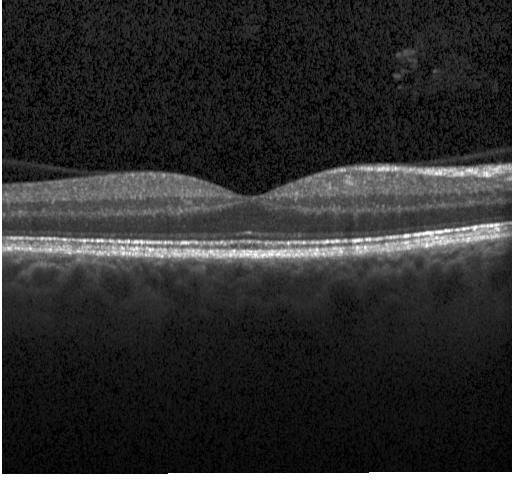 Instrument: Heidelberg Spectralis. Spectral-domain OCT. Retinal OCT B-scan. Through the macula — Dx: neither choroidal neovascularization, diabetic macular edema, nor drusen.